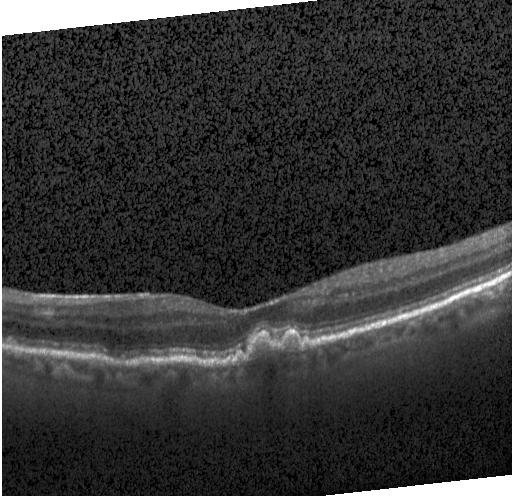
Assessment: drusen.